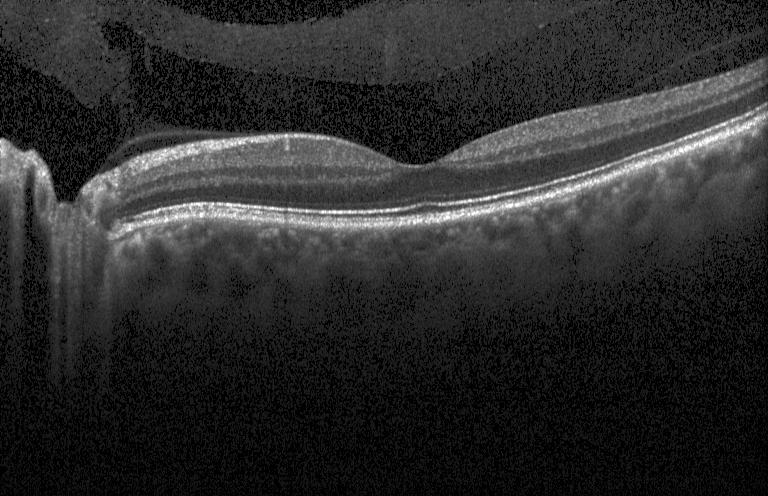

Horizontal scan through the fovea; optical coherence tomography scan; spectral-domain OCT; acquired on a Heidelberg Spectralis.
Finding: no choroidal neovascularization, diabetic macular edema, or drusen.